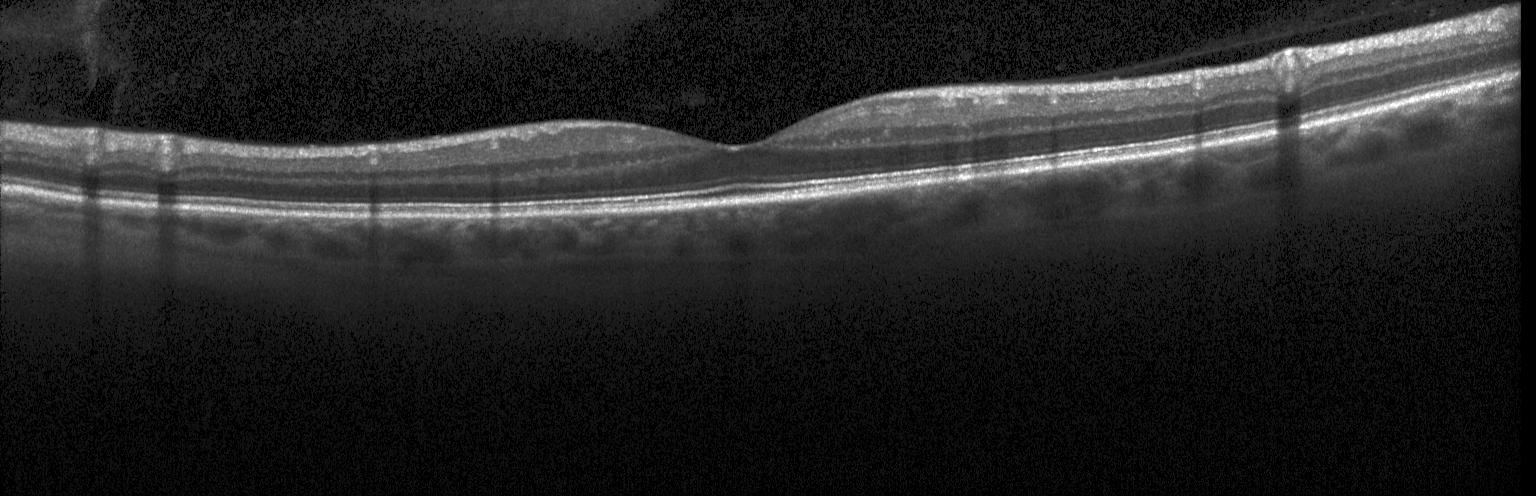 SD-OCT; Heidelberg Spectralis OCT system; retinal OCT cross-section — Impression: no choroidal neovascularization, no diabetic macular edema, and no drusen.